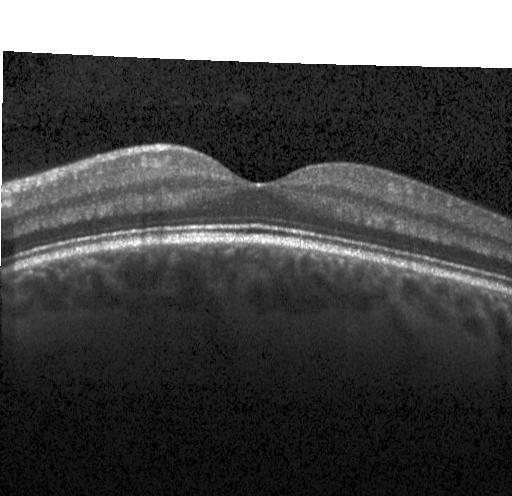
OCT scan showing no choroidal neovascularization, no diabetic macular edema, and no drusen.